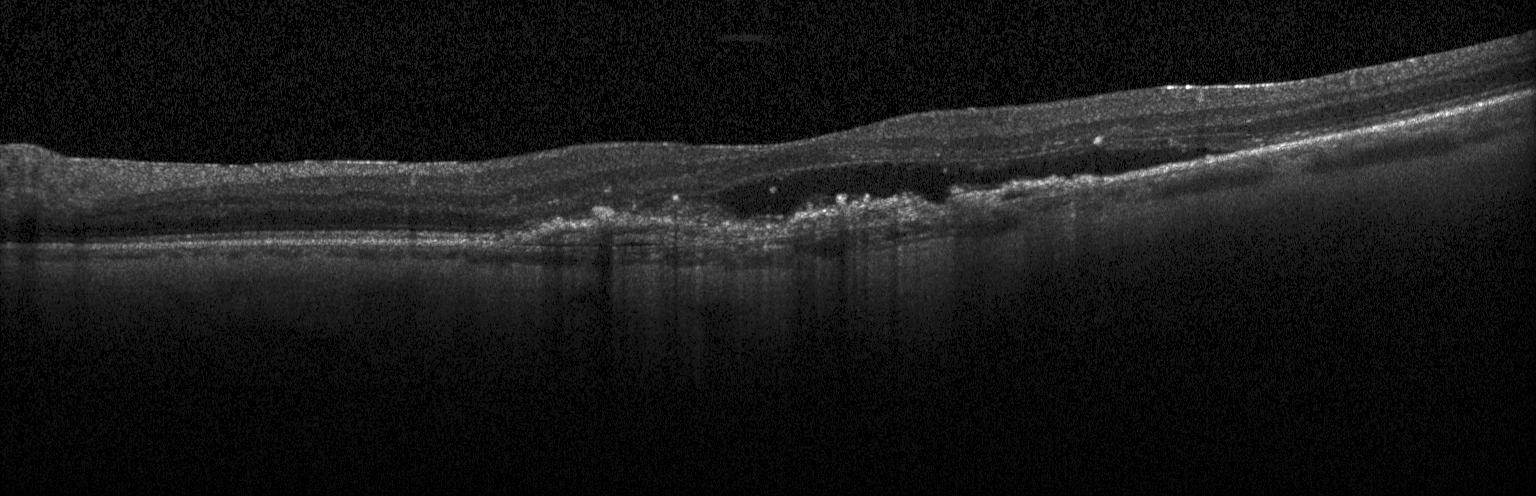

Retinal OCT B-scan. The scan shows a choroidal neovascular membrane.